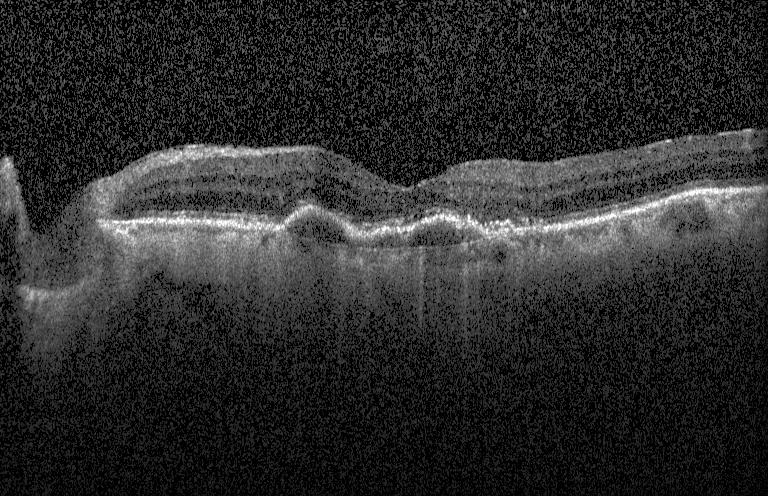 Spectral-domain OCT. Optical coherence tomography scan. Instrument: Heidelberg Spectralis. Impression: a choroidal neovascular membrane.